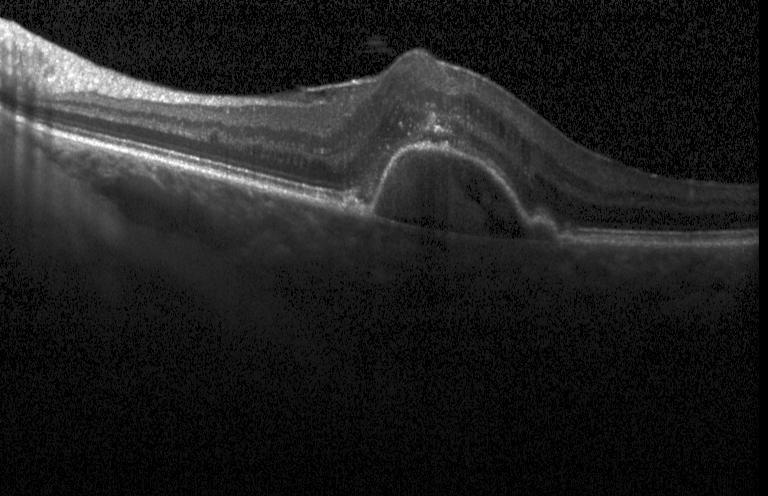 Finding: CNV.